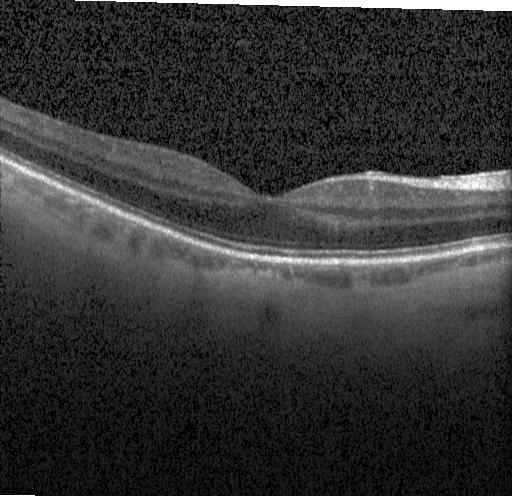 Retinal OCT B-scan. Heidelberg Spectralis — Assessment: no CNV, no DME, and no drusen.